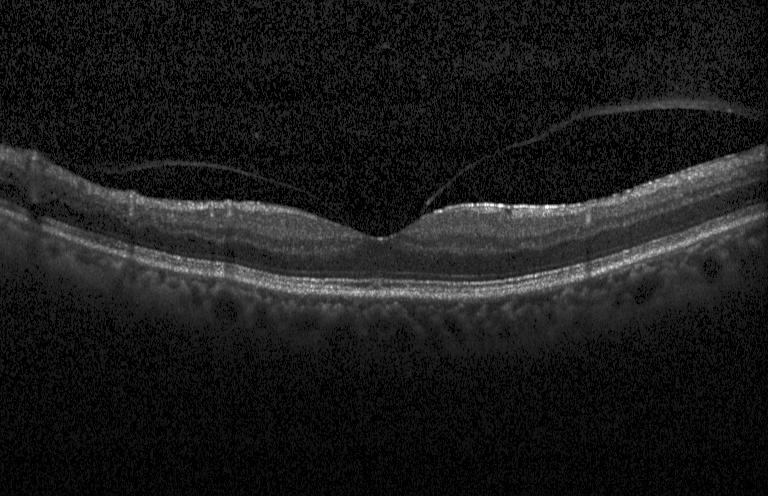

Impression: no choroidal neovascularization, diabetic macular edema, or drusen.